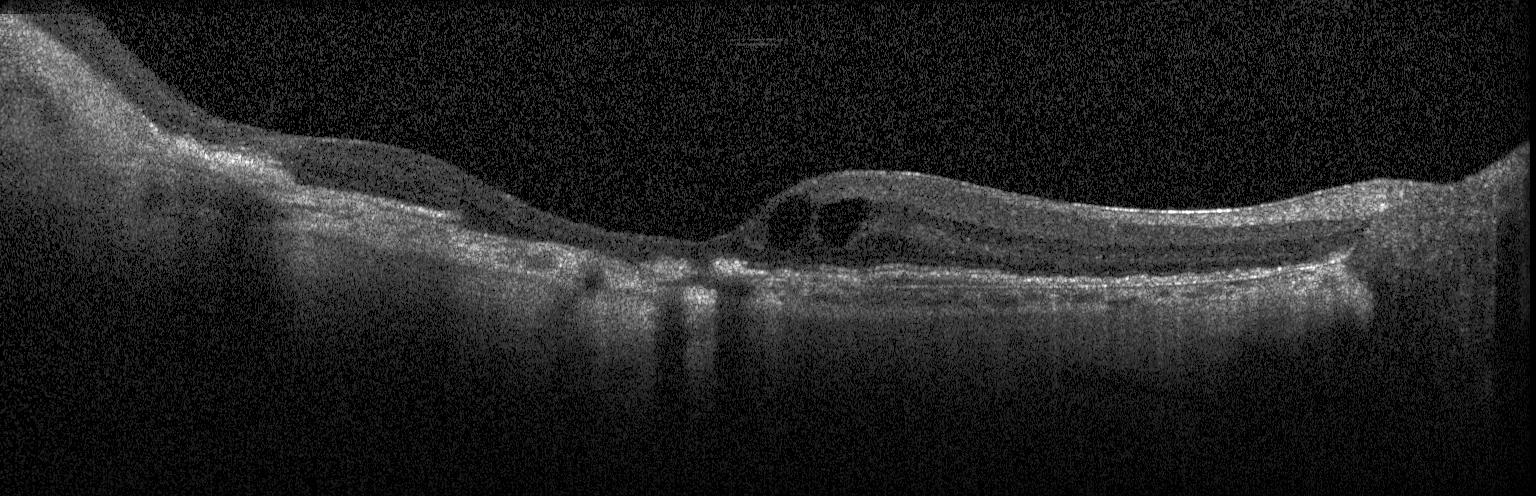

Retinal OCT B-scan
OCT finding: a choroidal neovascular membrane.